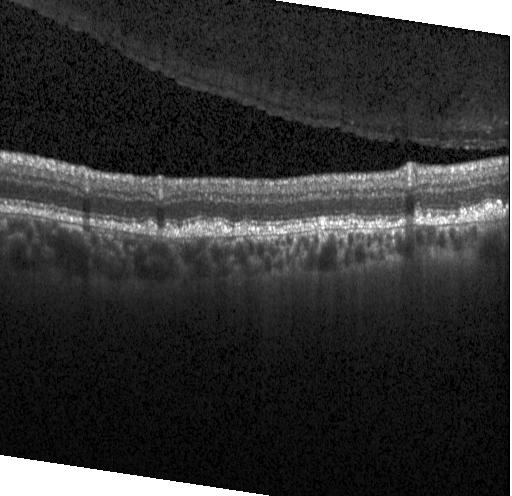 This B-scan demonstrates drusen.